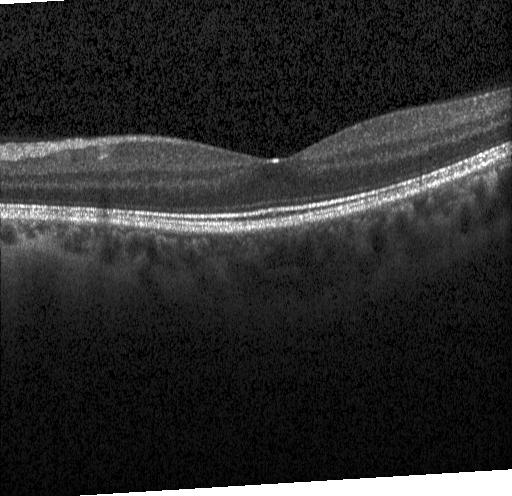
Dx: neither choroidal neovascularization, diabetic macular edema, nor drusen.